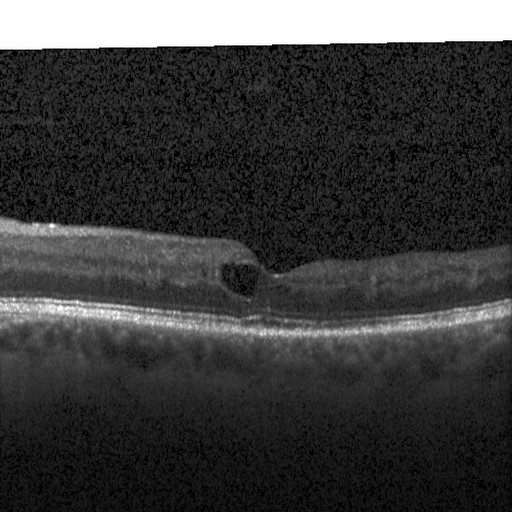

OCT finding: diabetic macular edema.